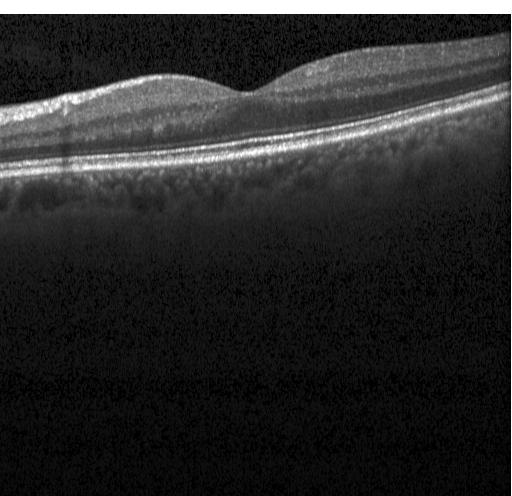

Retinal OCT cross-section. Diagnosis: no choroidal neovascularization, no diabetic macular edema, and no drusen.